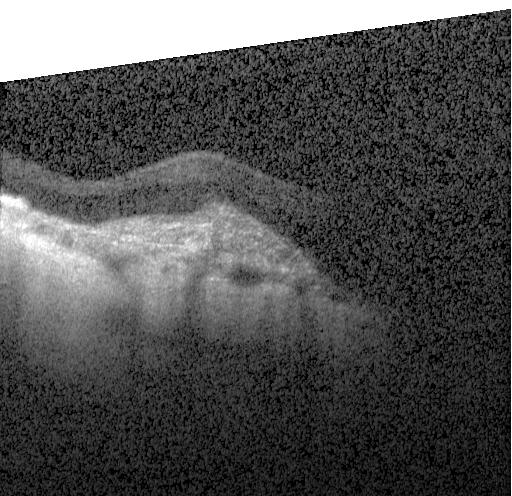 Retinal OCT B-scan — Macular OCT: a choroidal neovascular membrane.